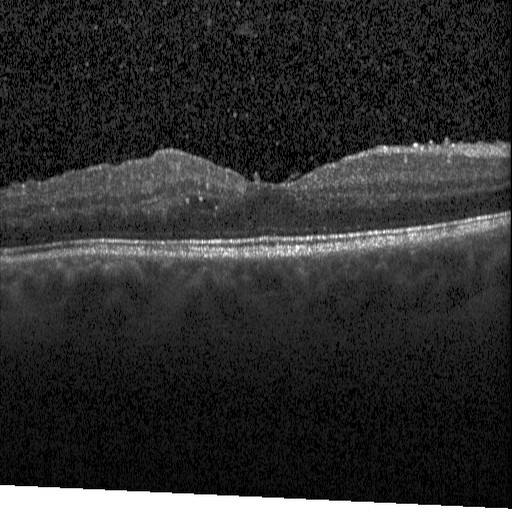 The scan shows DME.